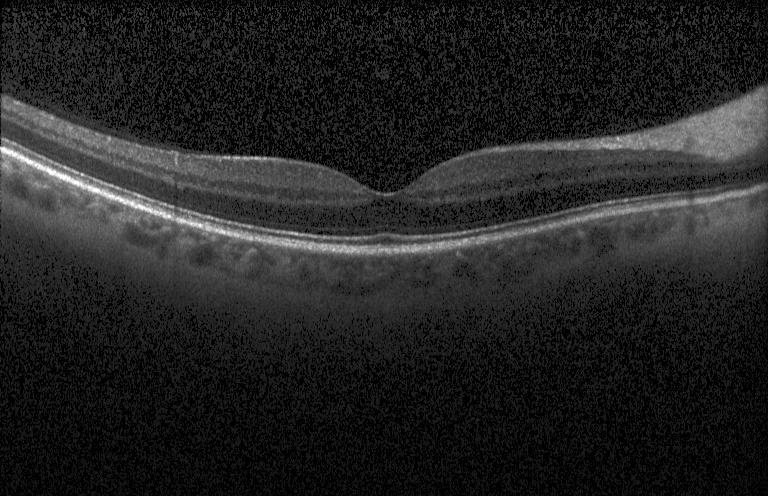
Optical coherence tomography scan · spectral-domain OCT. Finding: neither choroidal neovascularization, diabetic macular edema, nor drusen.